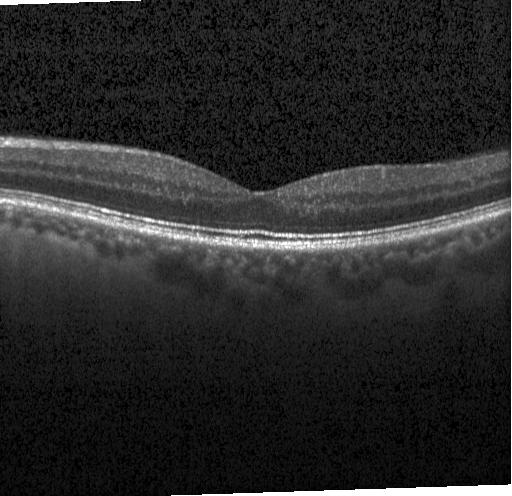

Horizontal scan through the fovea, optical coherence tomography scan, SD-OCT.
Finding: no evidence of choroidal neovascularization, diabetic macular edema, or drusen.